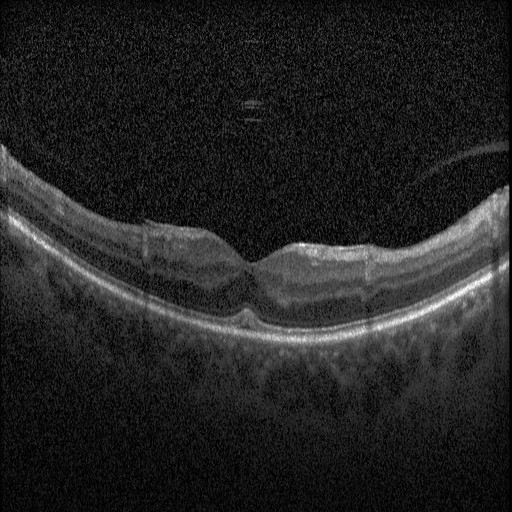
Optical coherence tomography B-scan. Assessment: diabetic macular edema (DME).